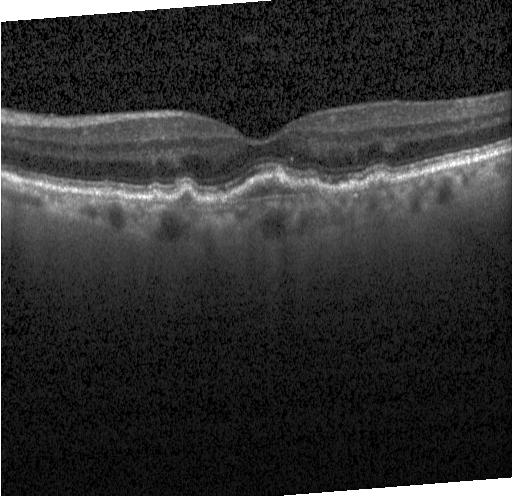
Acquired on a Heidelberg Spectralis, OCT B-scan, SD-OCT, macular scan.
Impression: a choroidal neovascular membrane.